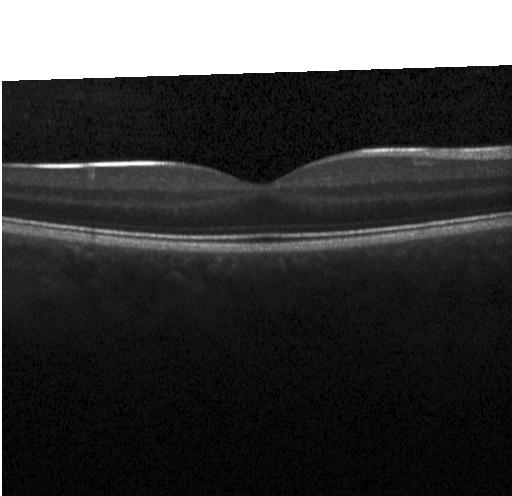
Heidelberg Spectralis OCT system. SD-OCT. Optical coherence tomography scan. Horizontal scan through the fovea.
Diagnosis: no CNV, DME, or drusen.